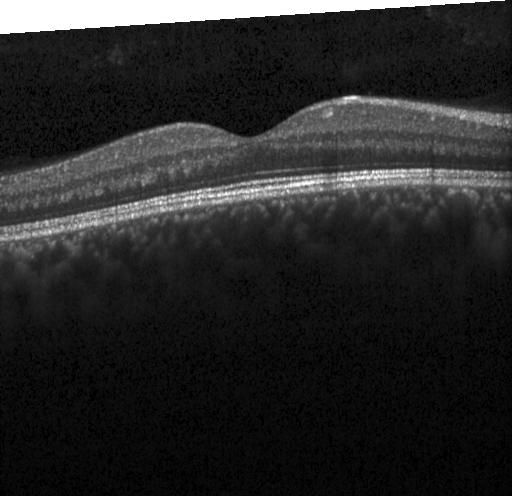 OCT B-scan, SD-OCT, Heidelberg Spectralis OCT system, horizontal scan through the fovea.
Diagnosis: no choroidal neovascularization, no diabetic macular edema, and no drusen.